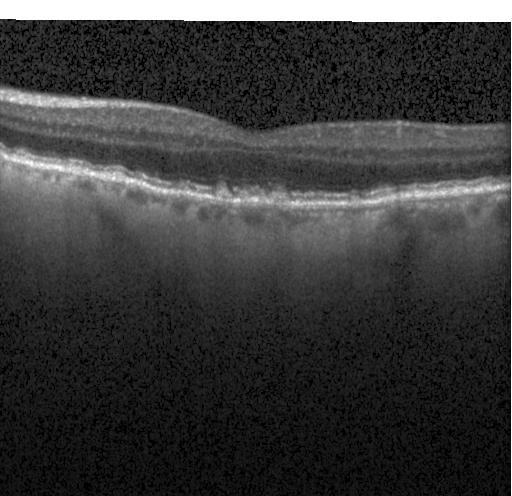 This B-scan demonstrates sub-RPE drusenoid deposits.